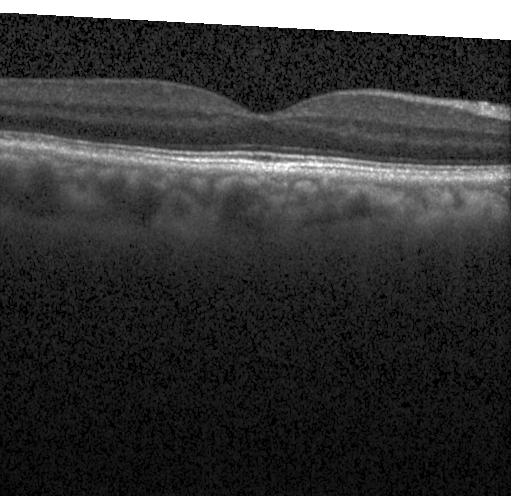
Optical coherence tomography B-scan · SD-OCT · through the macula. Dx: no evidence of CNV, DME, or drusen.